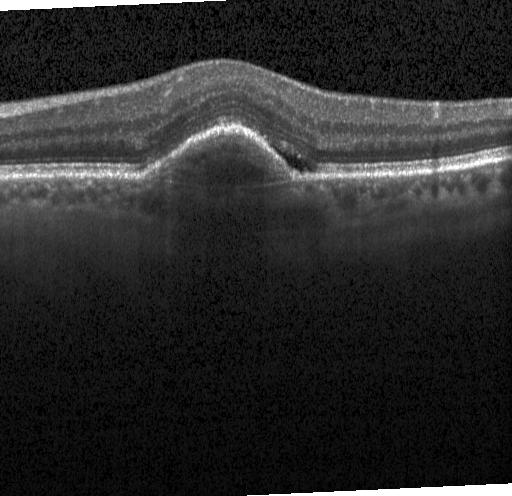 Spectral-domain OCT, OCT line scan, Heidelberg Spectralis OCT system.
The scan shows choroidal neovascularization.